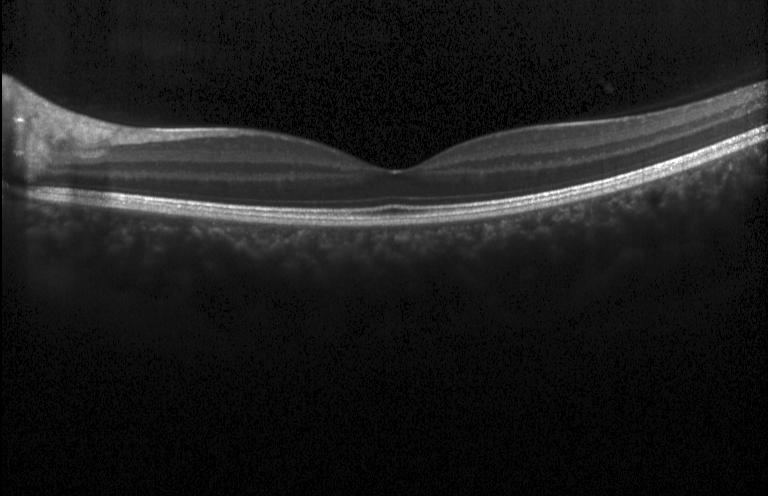

Spectral-domain optical coherence tomography; OCT B-scan. Finding: no evidence of choroidal neovascularization, diabetic macular edema, or drusen.